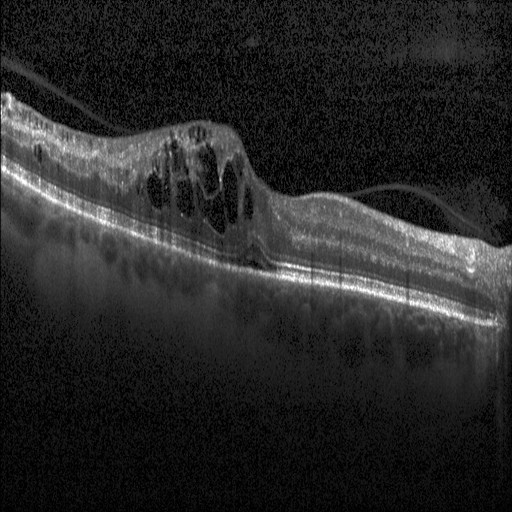

Retinal OCT cross-section showing diabetic macular edema.